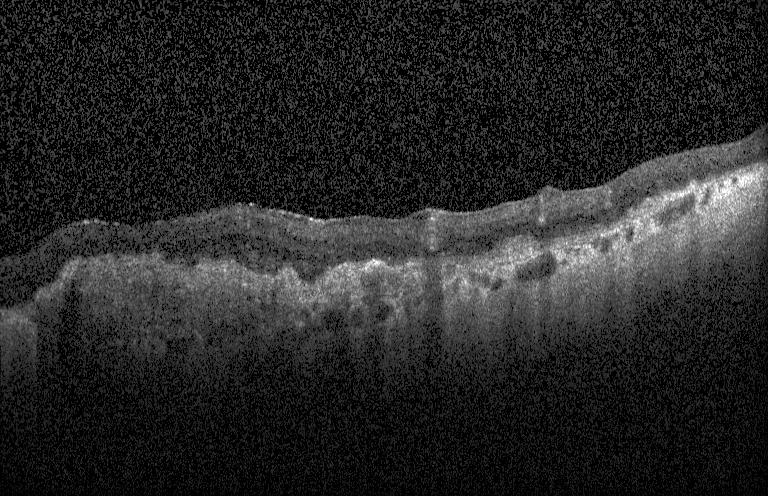
This B-scan demonstrates a choroidal neovascular membrane.